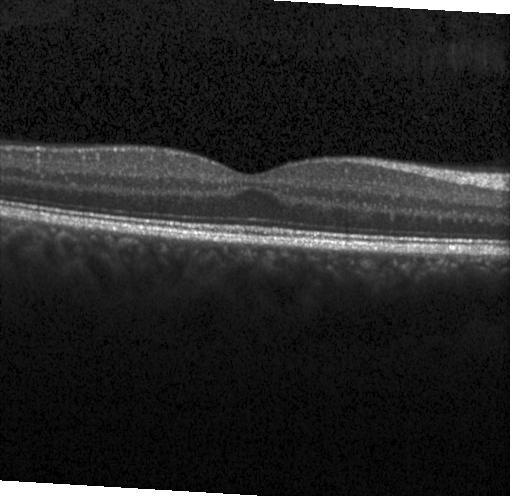

OCT finding: no choroidal neovascularization, no diabetic macular edema, and no drusen.